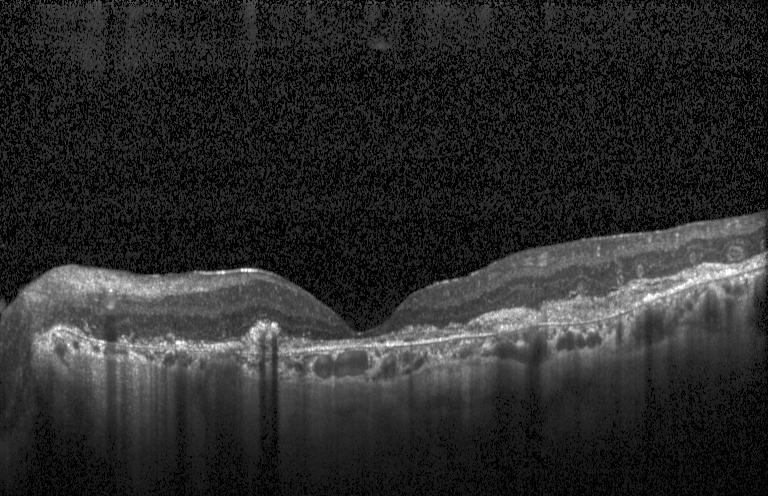 Centered on the fovea; optical coherence tomography B-scan; acquired on a Heidelberg Spectralis
Diagnosis: a choroidal neovascular membrane.